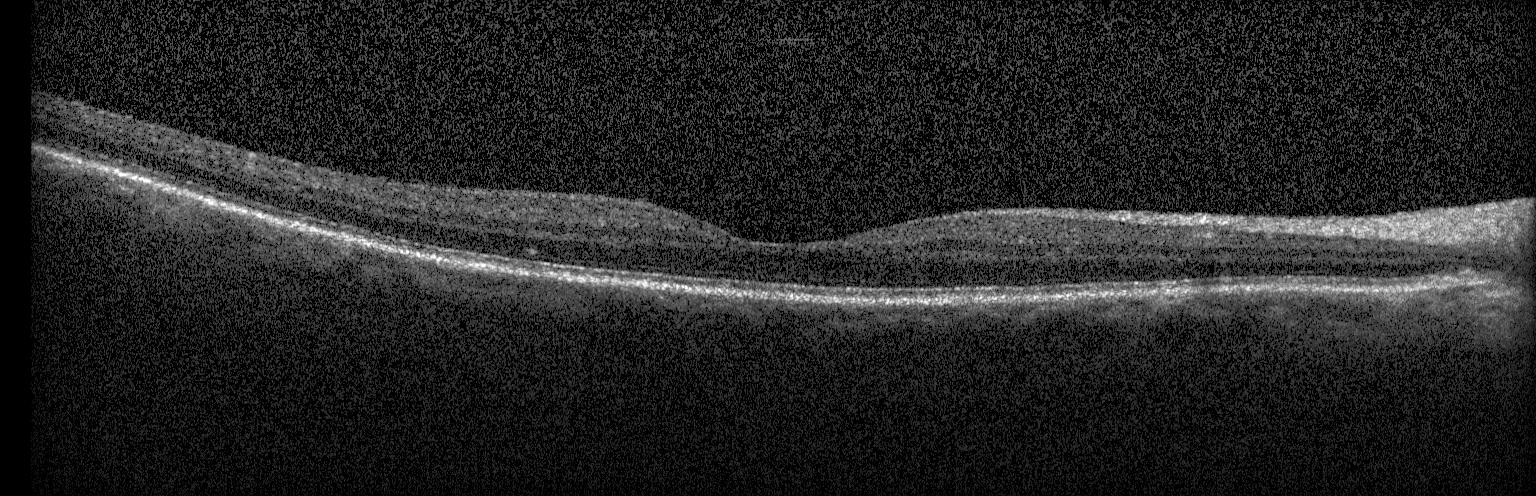 Heidelberg Spectralis · OCT B-scan · horizontal scan through the fovea. This B-scan demonstrates no evidence of CNV, DME, or drusen.